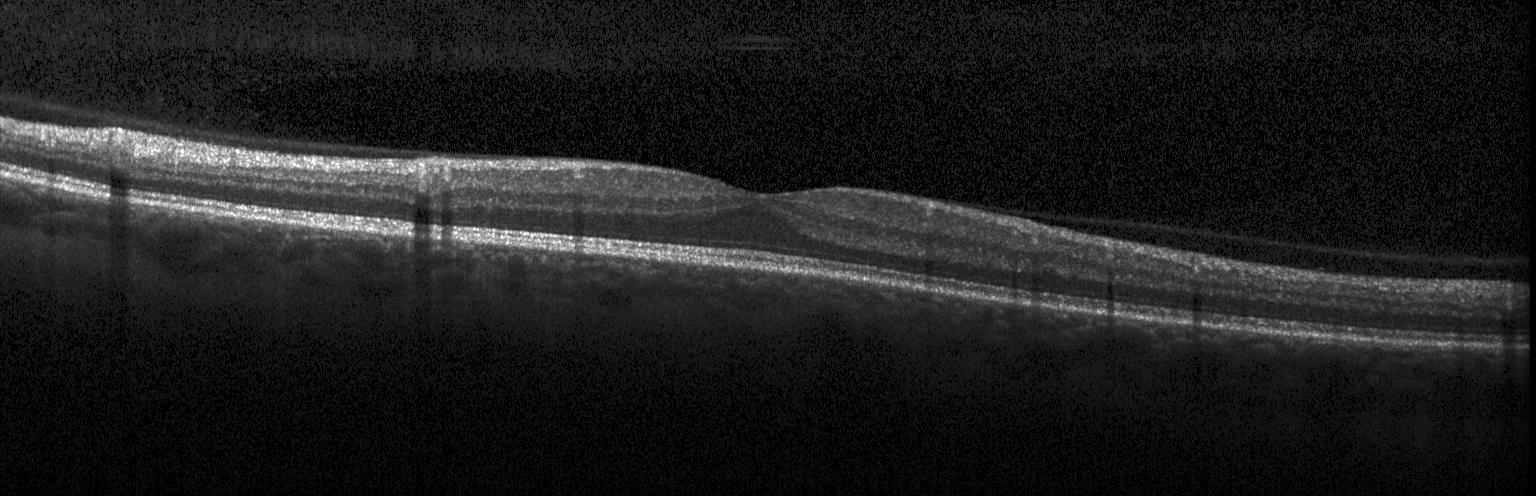

Retinal OCT cross-section.
Finding: no choroidal neovascularization, no diabetic macular edema, and no drusen.